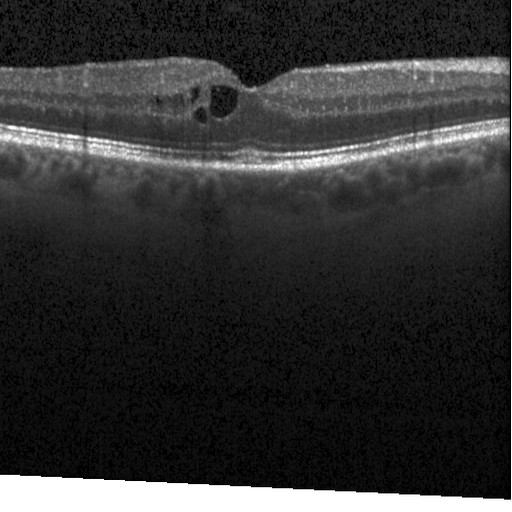

SD-OCT. Macular scan. Heidelberg Spectralis. Retinal OCT B-scan.
Impression: diabetic macular edema (DME).